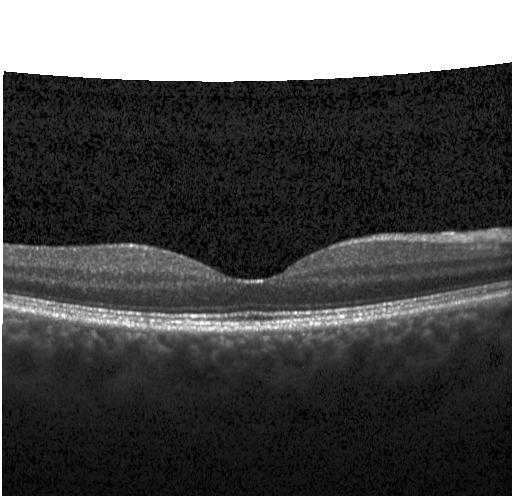 Macular OCT: no CNV, DME, or drusen.